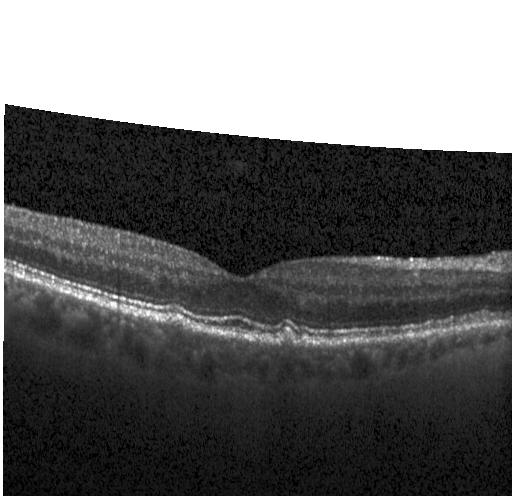
Retinal OCT cross-section. SD-OCT. Heidelberg Spectralis OCT system.
Diagnosis: drusen.